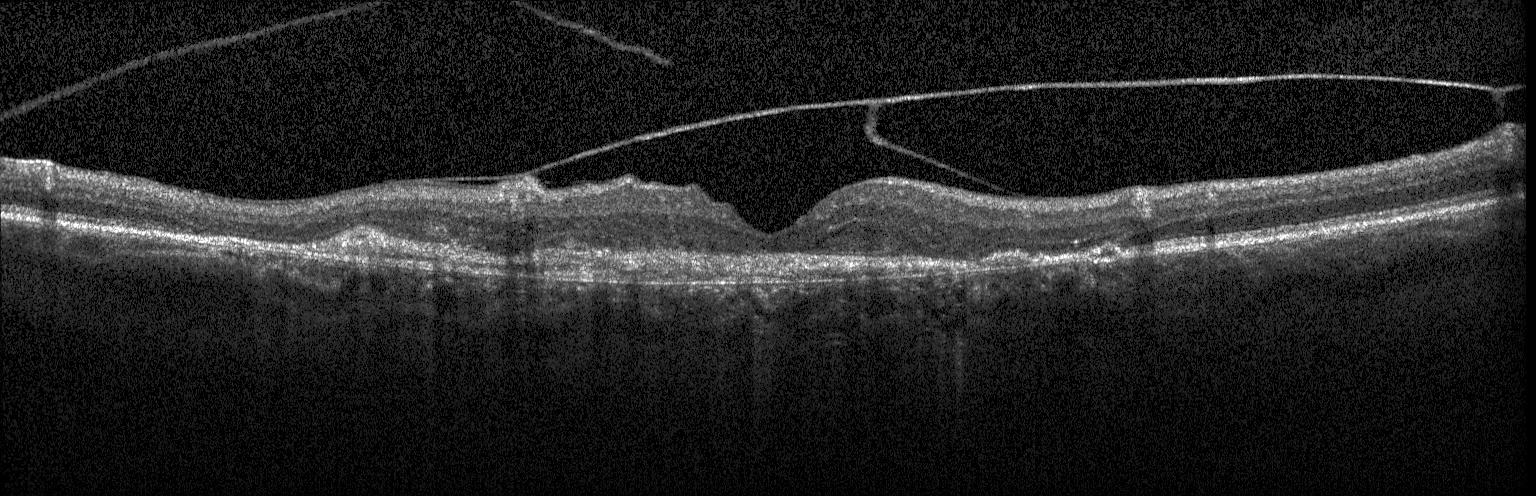

Macular OCT: a choroidal neovascular membrane.